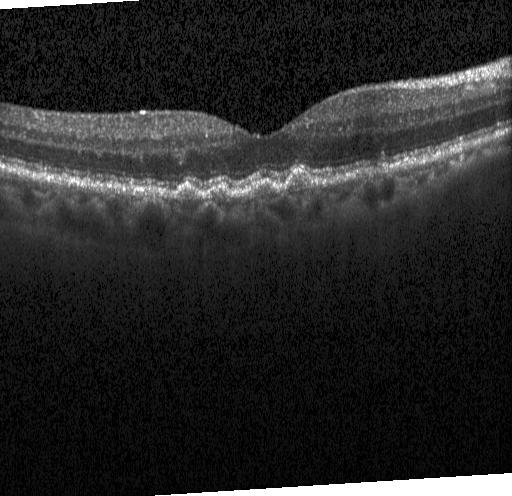 Spectral-domain optical coherence tomography, retinal OCT B-scan, through the macula.
This B-scan demonstrates sub-RPE drusenoid deposits.